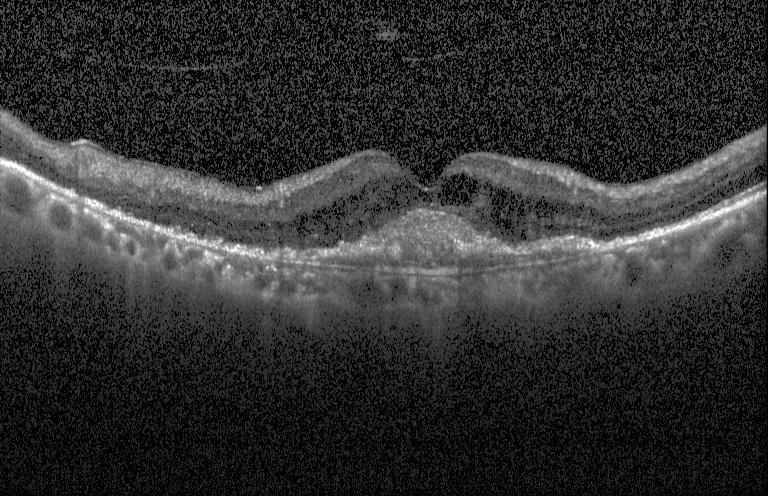
OCT B-scan showing a choroidal neovascular membrane.